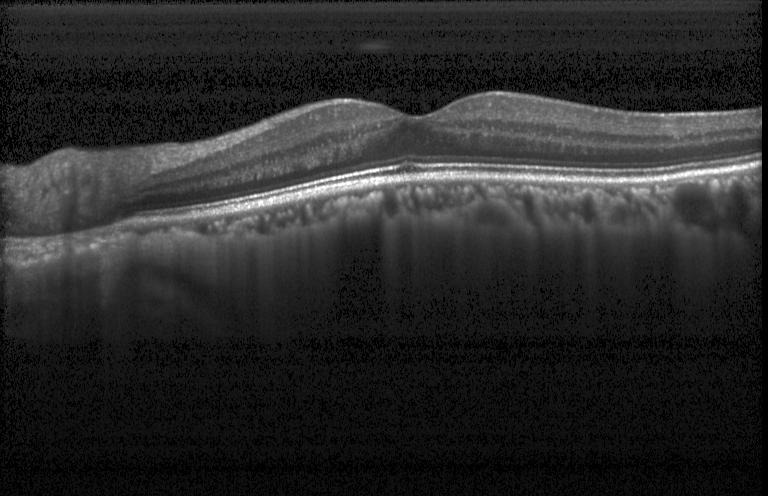

Fovea-centered, retinal OCT B-scan, SD-OCT, instrument: Heidelberg Spectralis — Finding: no evidence of choroidal neovascularization, diabetic macular edema, or drusen.